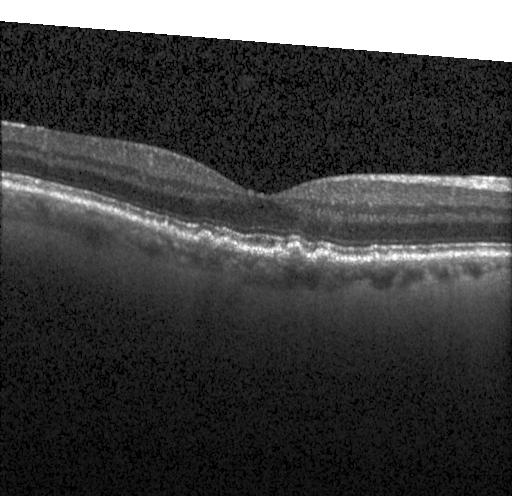
Macular OCT: drusen.